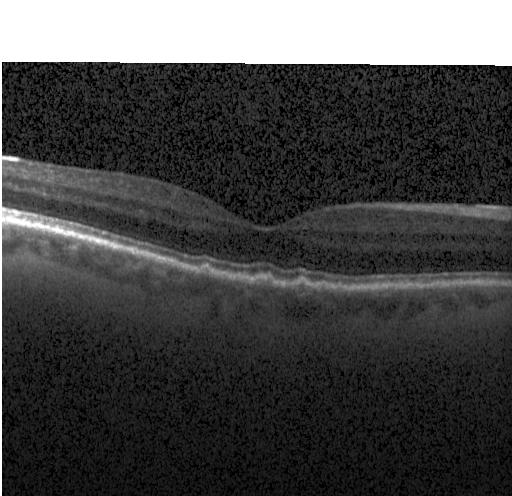 Multiple drusen.